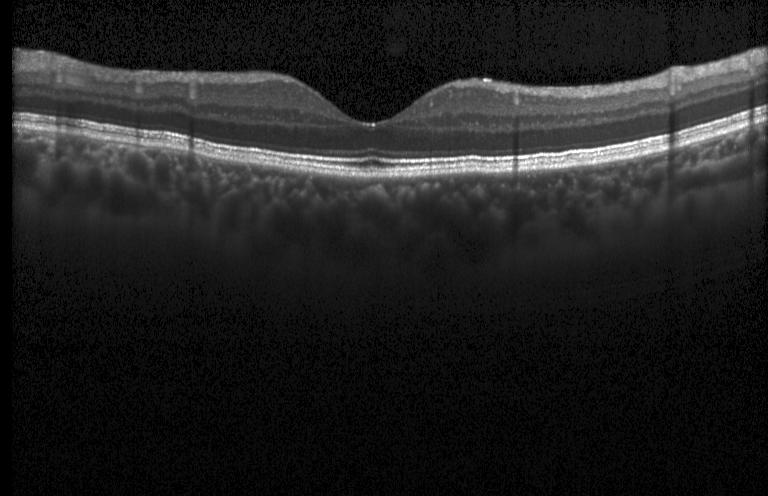
Optical coherence tomography B-scan. Impression: neither choroidal neovascularization, diabetic macular edema, nor drusen.